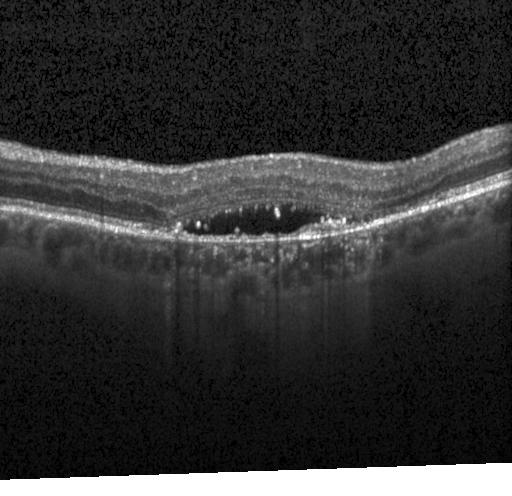
Spectral-domain OCT; retinal OCT B-scan
Diagnosis: CNV.